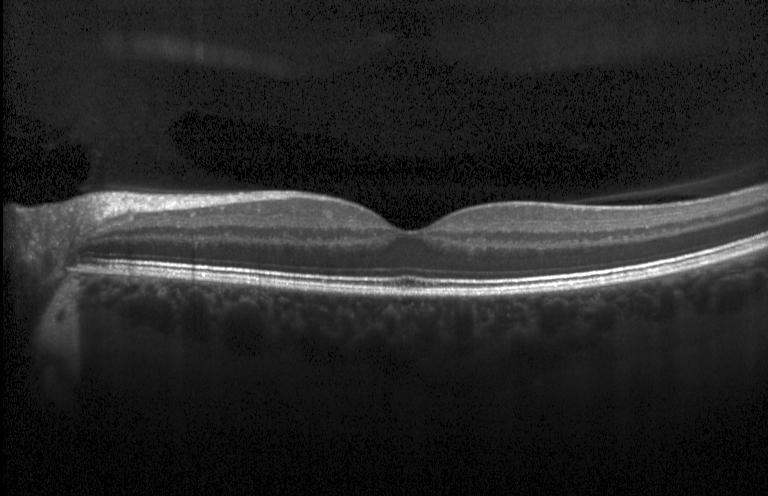
Optical coherence tomography scan
OCT finding: no CNV, DME, or drusen.